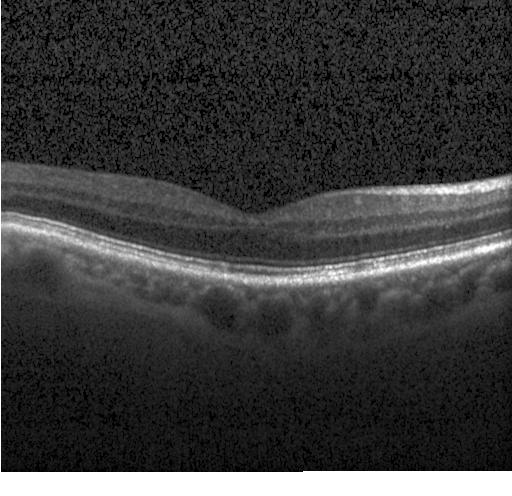

Dx: no CNV, no DME, and no drusen.